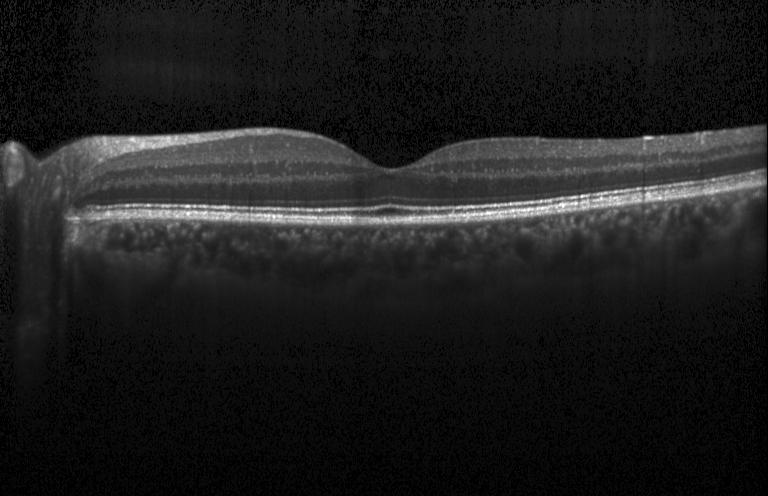
Finding: no choroidal neovascularization, no diabetic macular edema, and no drusen.